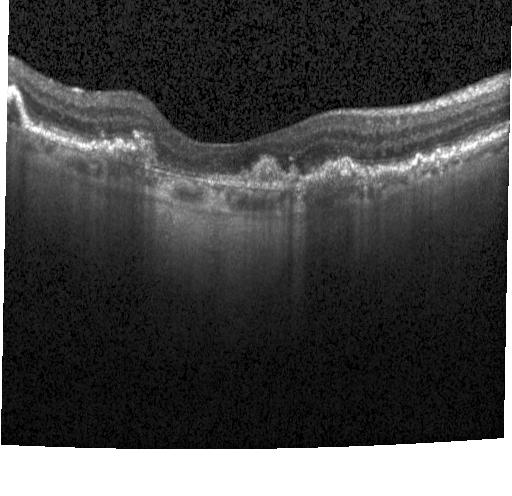 Instrument: Heidelberg Spectralis; optical coherence tomography B-scan; through the macula — Impression: a choroidal neovascular membrane.